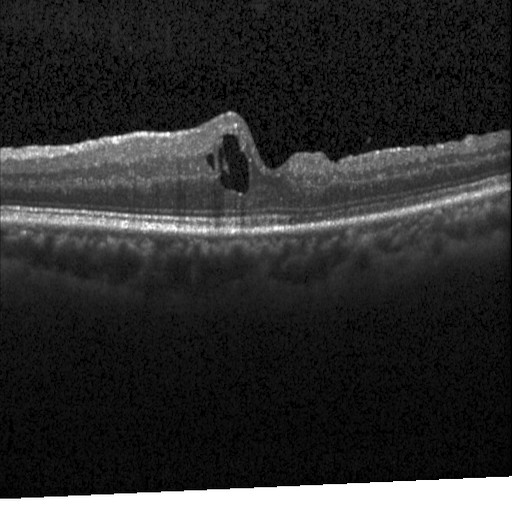

Heidelberg Spectralis OCT system, macular scan, SD-OCT, OCT B-scan
OCT finding: DME.